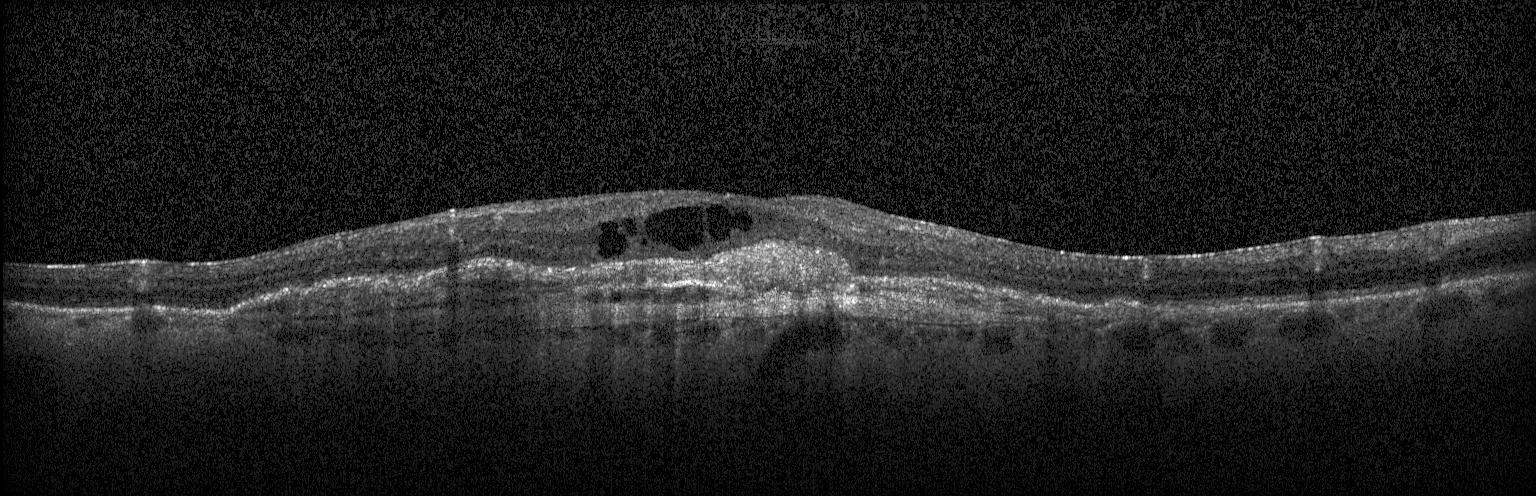 A choroidal neovascular membrane.